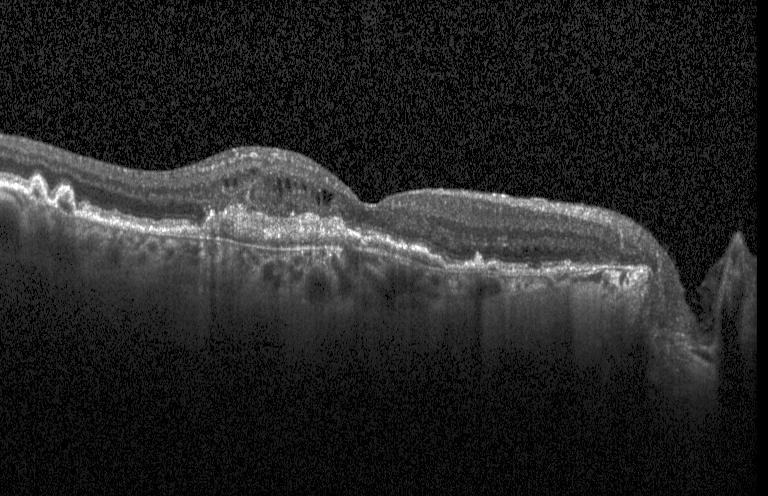

Retinal OCT cross-section showing a choroidal neovascular membrane.